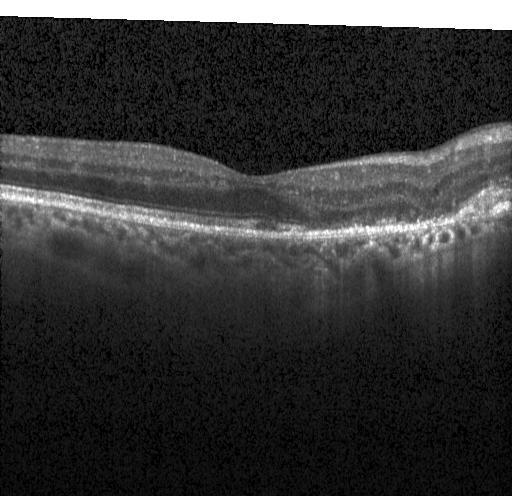
Spectral-domain optical coherence tomography; OCT line scan; instrument: Heidelberg Spectralis
Diagnosis: choroidal neovascularization.